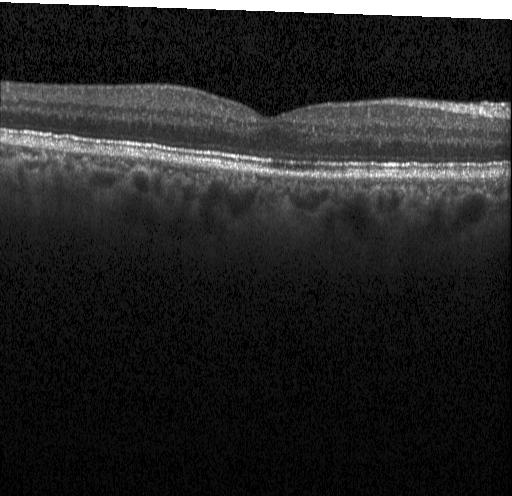
OCT line scan. Through the macula. Spectral-domain OCT. Instrument: Heidelberg Spectralis — Macular OCT: no choroidal neovascularization, no diabetic macular edema, and no drusen.